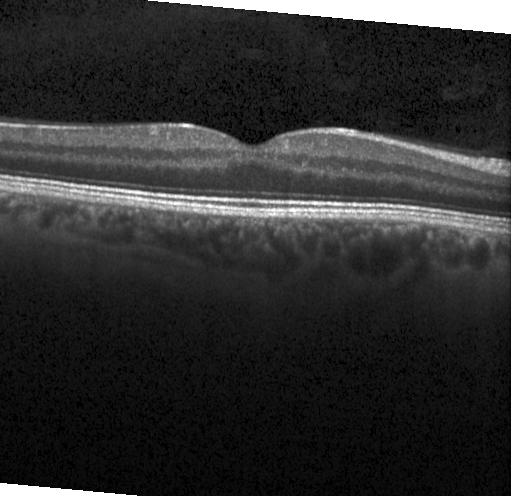 The scan shows no evidence of CNV, DME, or drusen.